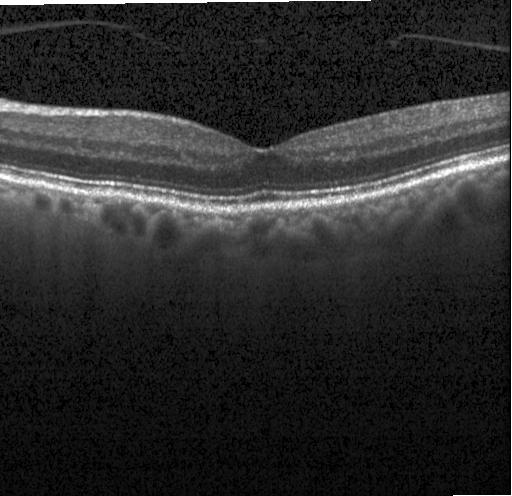

Spectral-domain optical coherence tomography, instrument: Heidelberg Spectralis, through the macula, OCT line scan — Assessment: no choroidal neovascularization, no diabetic macular edema, and no drusen.